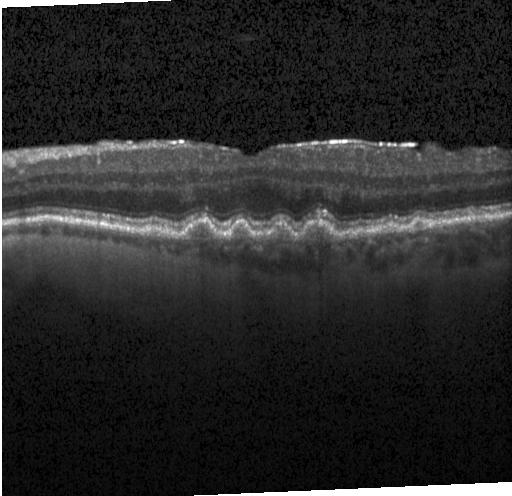

Heidelberg Spectralis. Optical coherence tomography scan. Spectral-domain OCT. Fovea-centered.
Drusen.